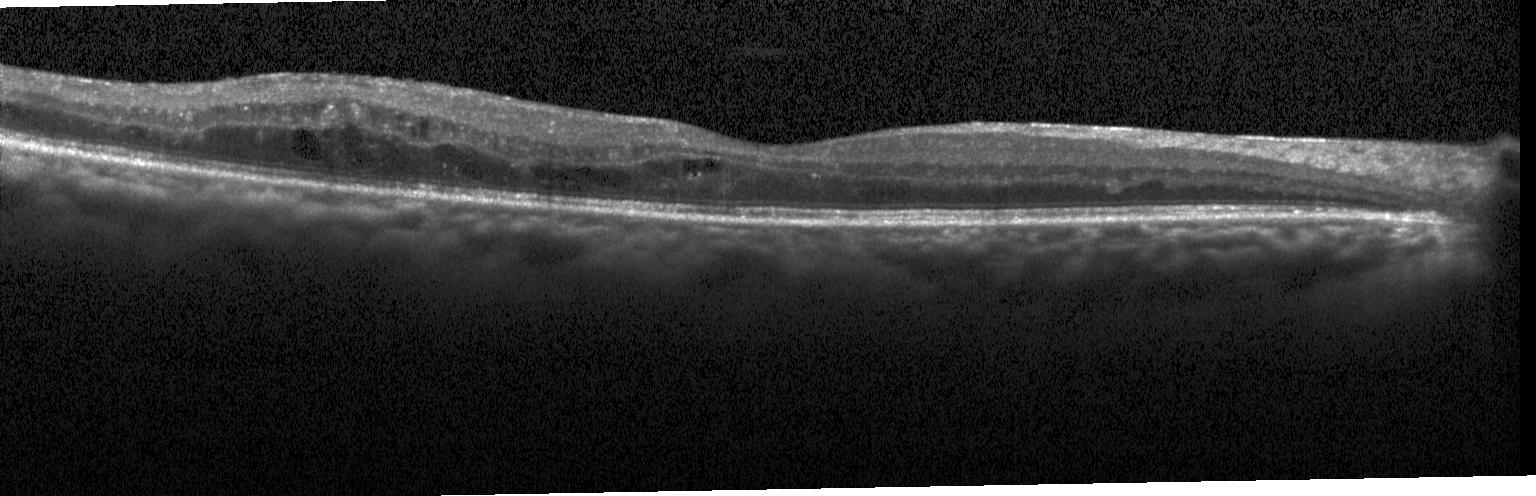 This B-scan demonstrates DME.